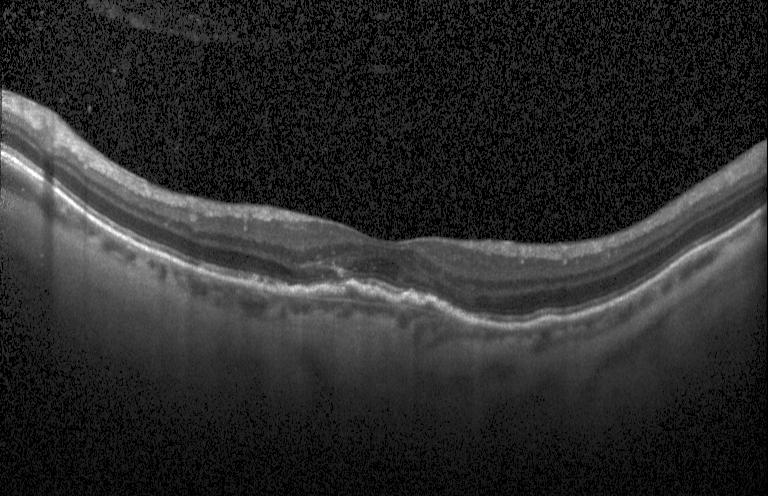
Assessment: a choroidal neovascular membrane.